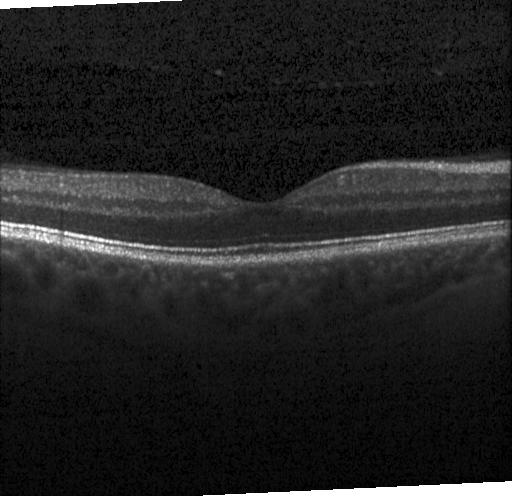 SD-OCT. OCT line scan. Through the macula. Instrument: Heidelberg Spectralis — Finding: no choroidal neovascularization, diabetic macular edema, or drusen.